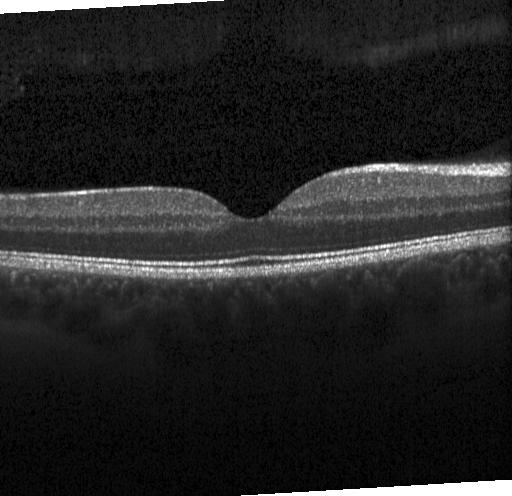

This B-scan demonstrates neither choroidal neovascularization, diabetic macular edema, nor drusen.